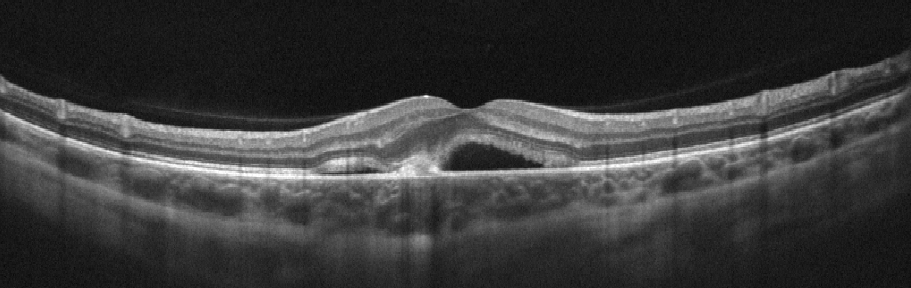
Fovea-centered; Optovue Avanti RTVue XR; optical coherence tomography B-scan
OCT finding: age-related macular degeneration.